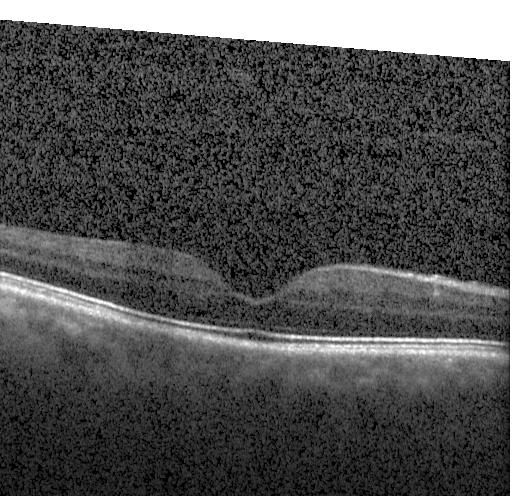

Macular OCT demonstrating no evidence of choroidal neovascularization, diabetic macular edema, or drusen.